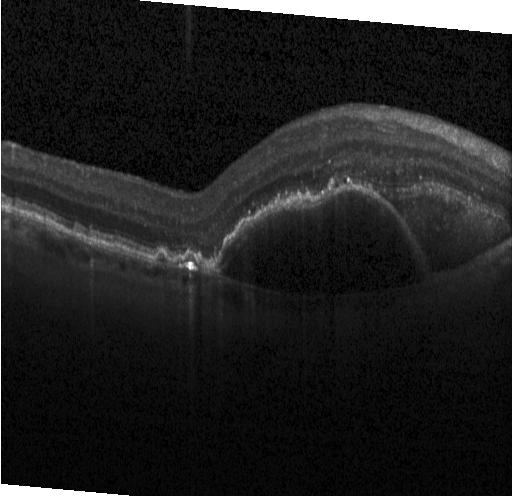 Instrument: Heidelberg Spectralis. OCT line scan. Spectral-domain OCT — Finding: choroidal neovascularization (CNV).